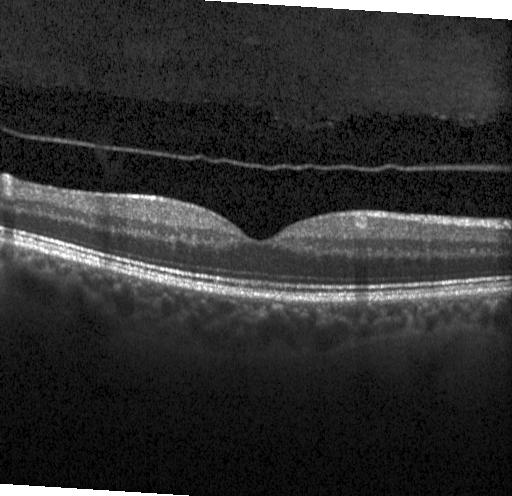
Diagnosis: no evidence of CNV, DME, or drusen.